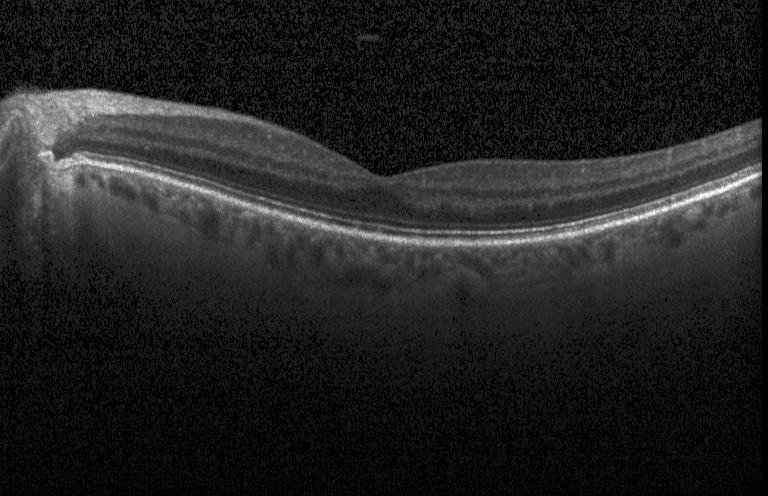
Centered on the fovea, spectral-domain OCT, optical coherence tomography B-scan, Heidelberg Spectralis. Impression: no evidence of CNV, DME, or drusen.